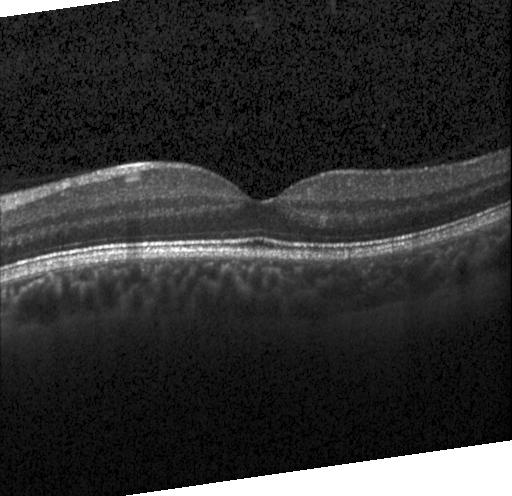
Dx: no choroidal neovascularization, diabetic macular edema, or drusen.